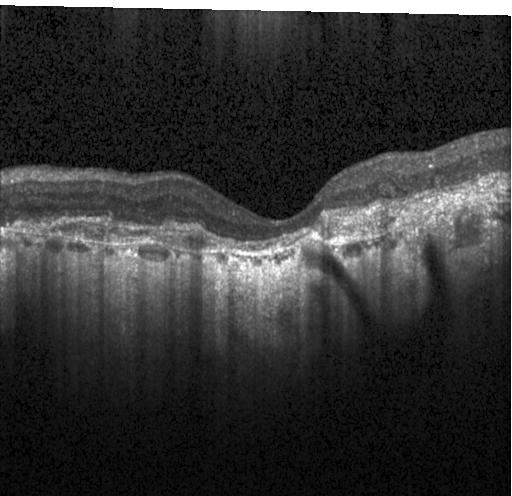 Fovea-centered; retinal OCT B-scan; spectral-domain optical coherence tomography; instrument: Heidelberg Spectralis.
The scan shows a choroidal neovascular membrane.